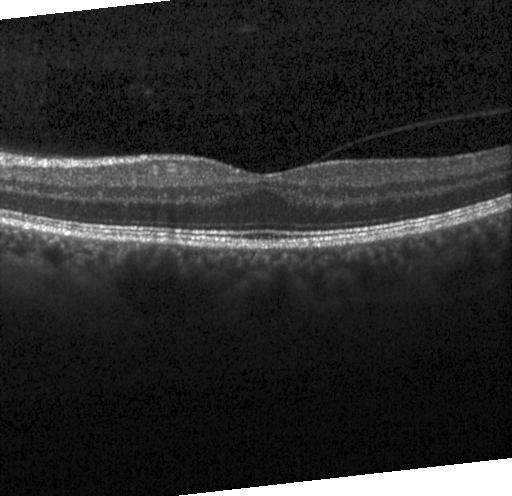

Retinal OCT B-scan.
Finding: no choroidal neovascularization, diabetic macular edema, or drusen.